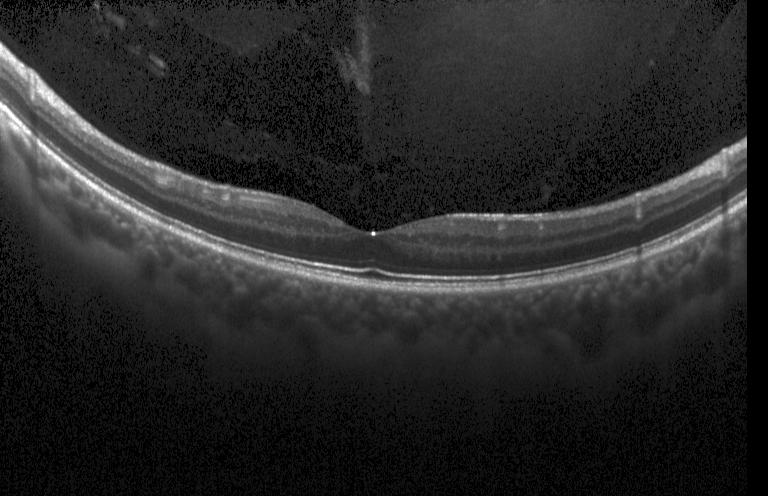
Assessment: no CNV, DME, or drusen.